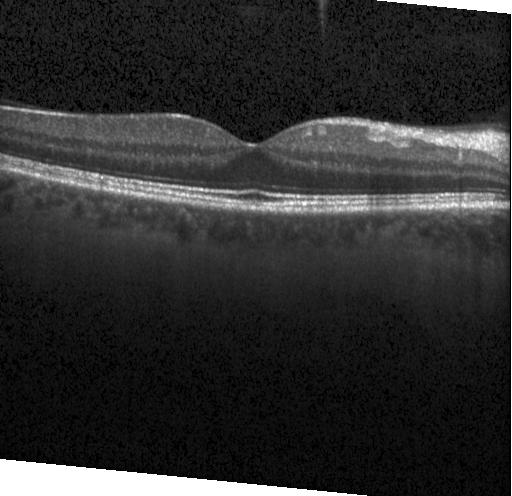 SD-OCT. Heidelberg Spectralis. OCT B-scan. Centered on the fovea. No choroidal neovascularization, no diabetic macular edema, and no drusen.